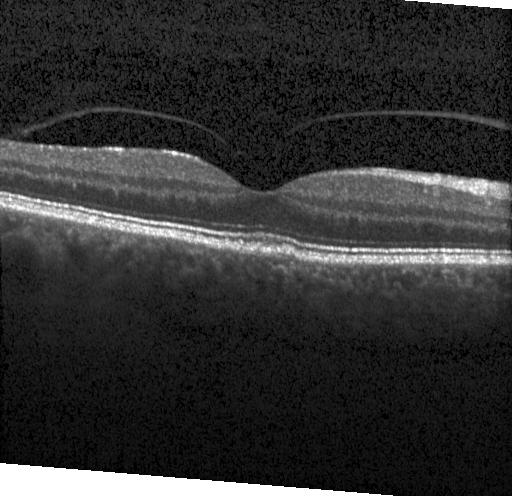
Macular scan, optical coherence tomography scan.
Assessment: drusen.